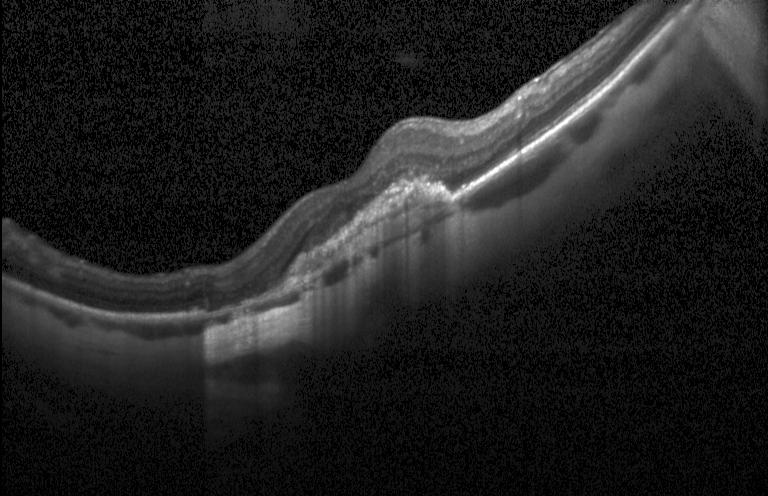

Diagnosis: a choroidal neovascular membrane.